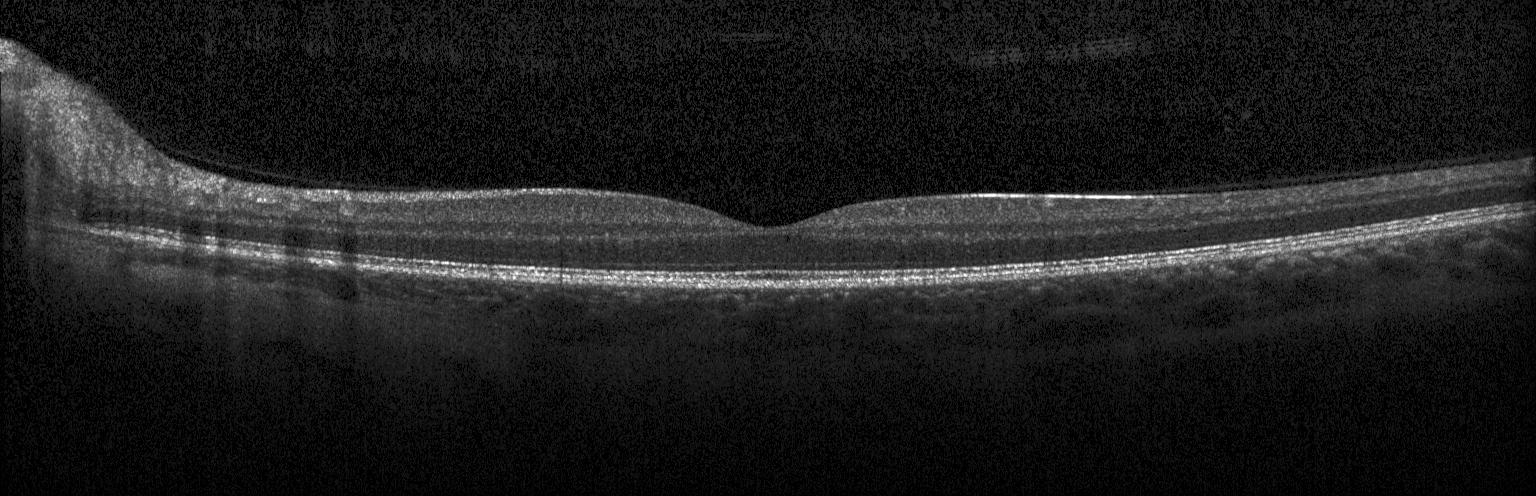

Finding: no evidence of CNV, DME, or drusen.